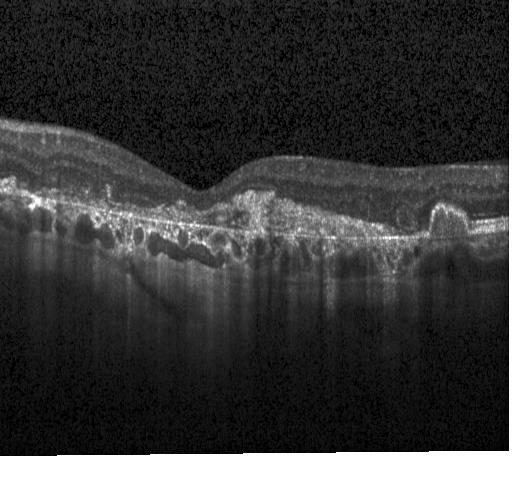

Finding: a choroidal neovascular membrane.